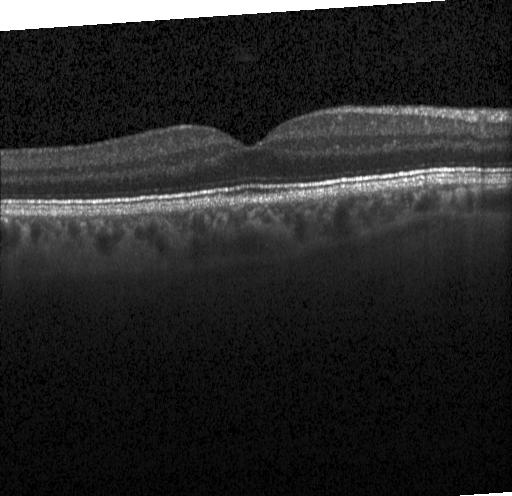
Retinal OCT cross-section showing no CNV, no DME, and no drusen.